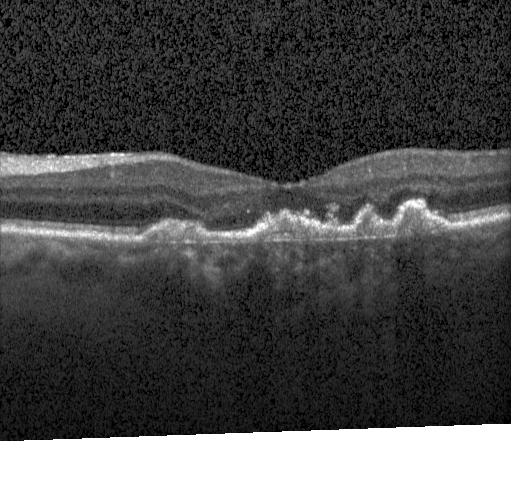 Macular OCT: choroidal neovascularization (CNV).